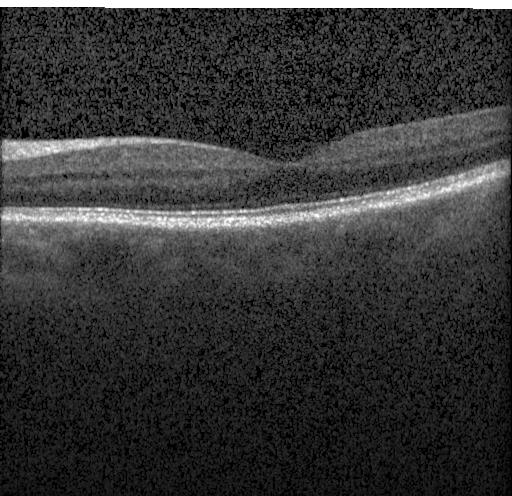

OCT line scan.
Finding: no choroidal neovascularization, diabetic macular edema, or drusen.